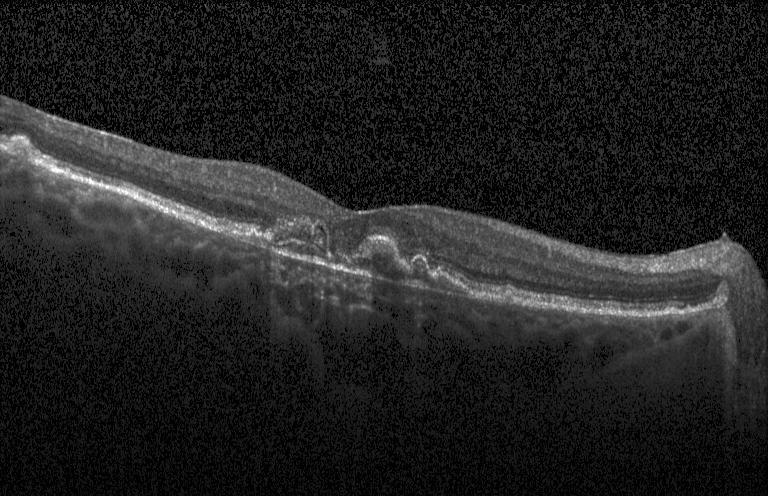

This B-scan demonstrates a choroidal neovascular membrane.